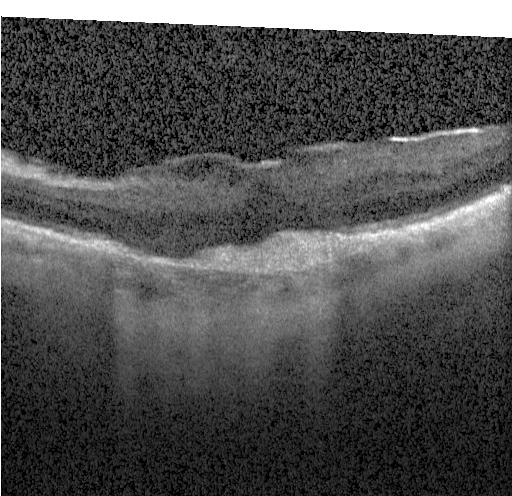
This B-scan demonstrates a choroidal neovascular membrane.